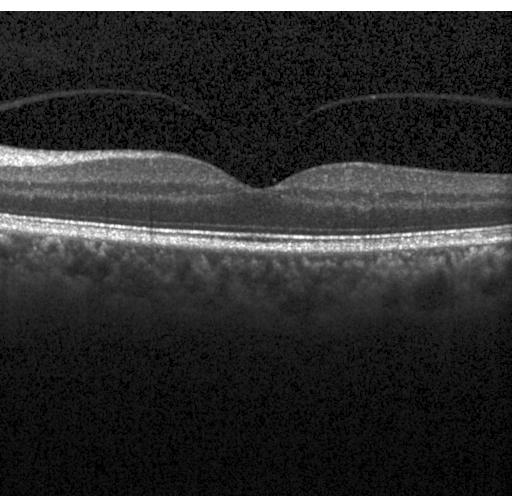
Retinal OCT B-scan.
Diagnosis: no choroidal neovascularization, no diabetic macular edema, and no drusen.